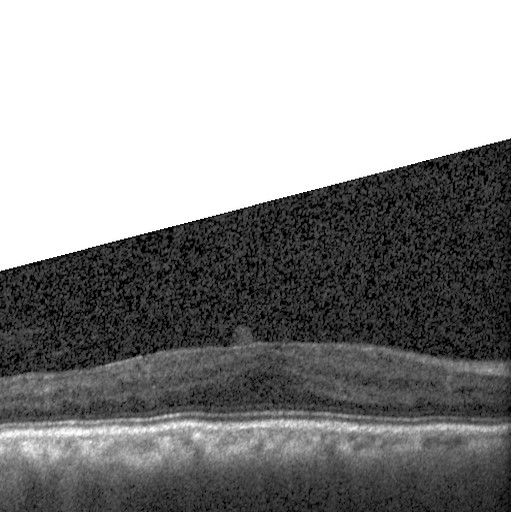
OCT B-scan; spectral-domain OCT; Heidelberg Spectralis OCT system
Impression: DME.